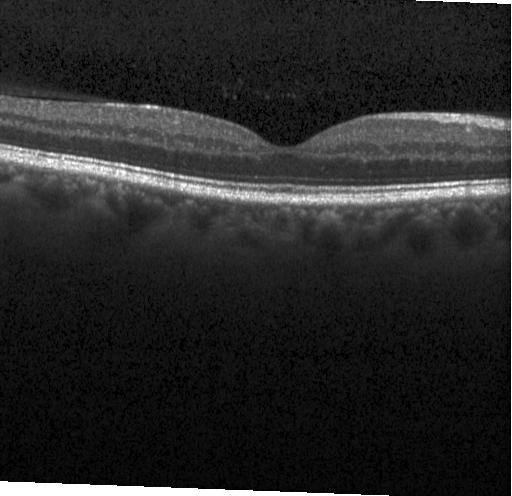
SD-OCT. Retinal OCT B-scan. Heidelberg Spectralis OCT system
This B-scan demonstrates no evidence of choroidal neovascularization, diabetic macular edema, or drusen.